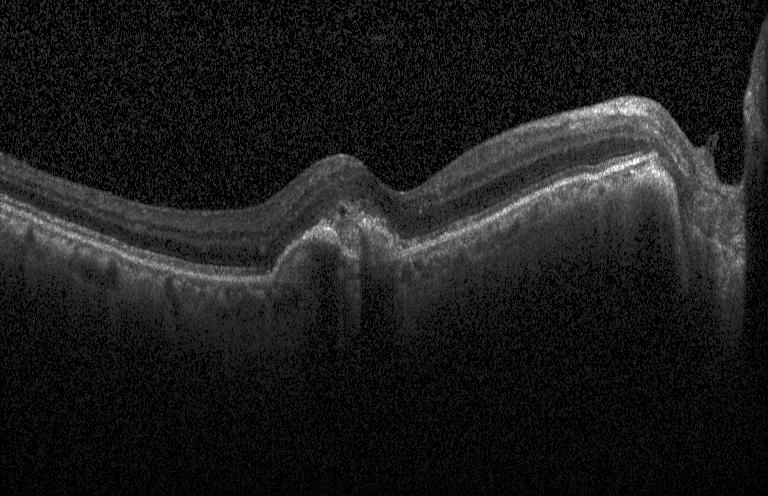
OCT line scan — Macular OCT: choroidal neovascularization.